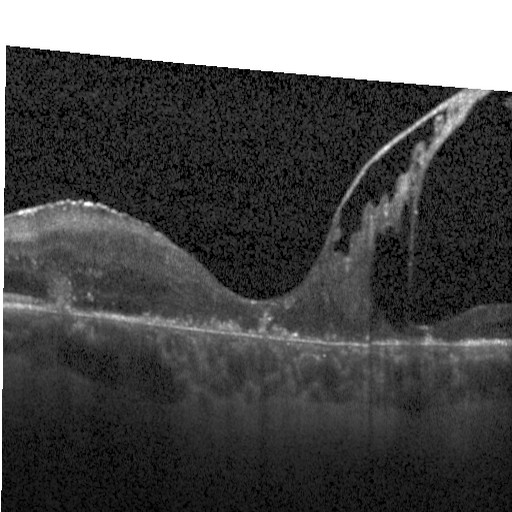
OCT B-scan, spectral-domain optical coherence tomography, instrument: Heidelberg Spectralis — Impression: diabetic macular edema (DME).